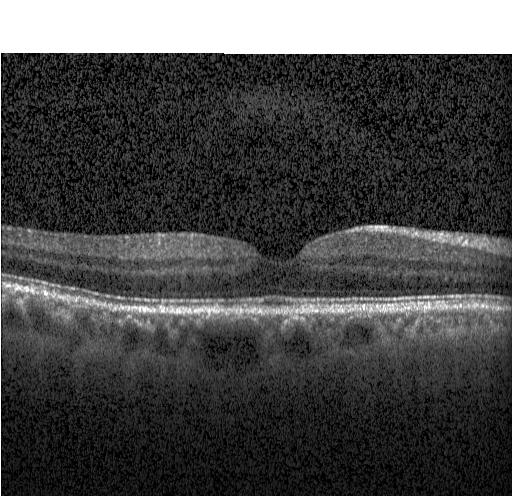

Optical coherence tomography B-scan · spectral-domain optical coherence tomography.
Finding: neither choroidal neovascularization, diabetic macular edema, nor drusen.